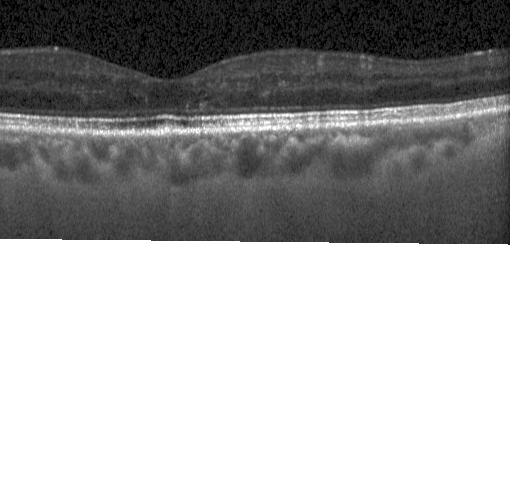

Spectral-domain OCT · fovea-centered · Heidelberg Spectralis · OCT B-scan
Diagnosis: no evidence of choroidal neovascularization, diabetic macular edema, or drusen.